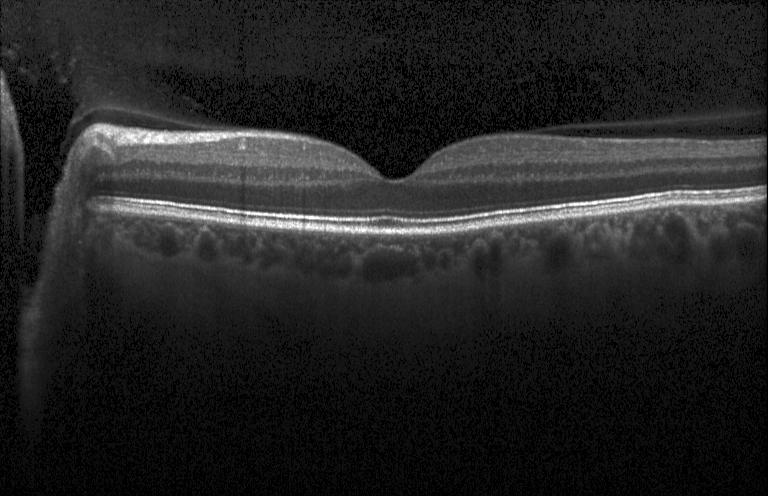
Spectral-domain optical coherence tomography; optical coherence tomography scan; fovea-centered; Heidelberg Spectralis
Finding: neither choroidal neovascularization, diabetic macular edema, nor drusen.